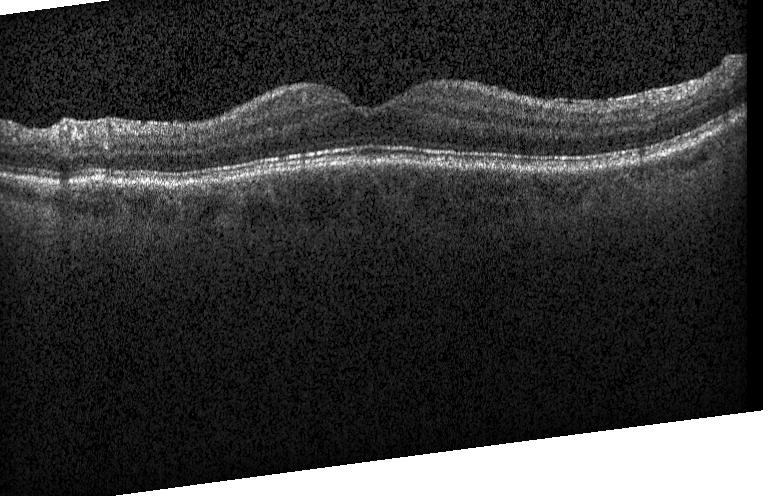

Instrument: Heidelberg Spectralis · centered on the fovea · optical coherence tomography B-scan · spectral-domain OCT — This B-scan demonstrates no evidence of CNV, DME, or drusen.